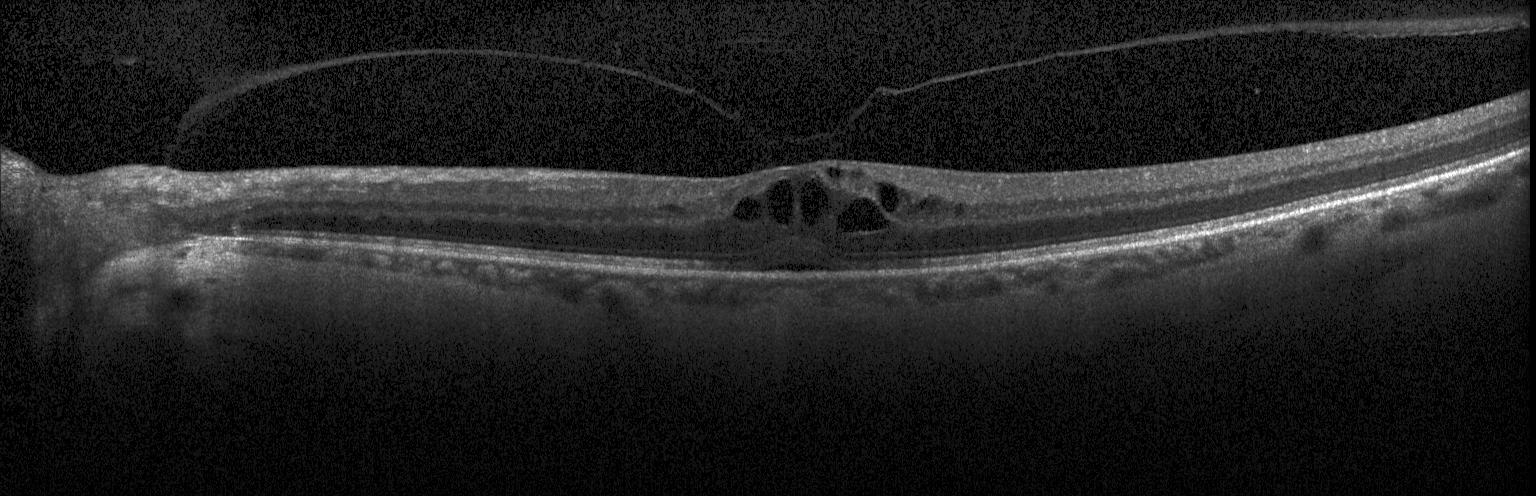 Dx: diabetic macular edema.